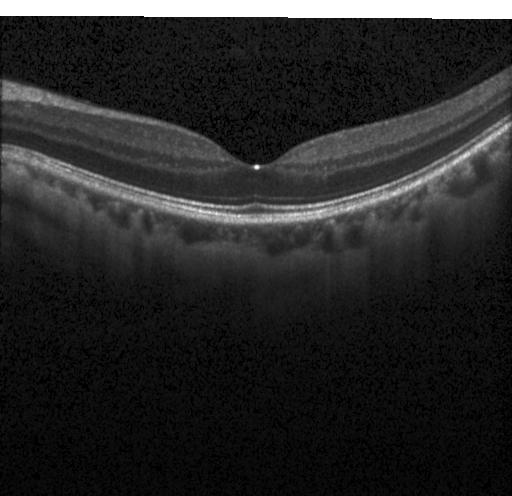 Spectral-domain optical coherence tomography. Retinal OCT cross-section.
Impression: no choroidal neovascularization, no diabetic macular edema, and no drusen.